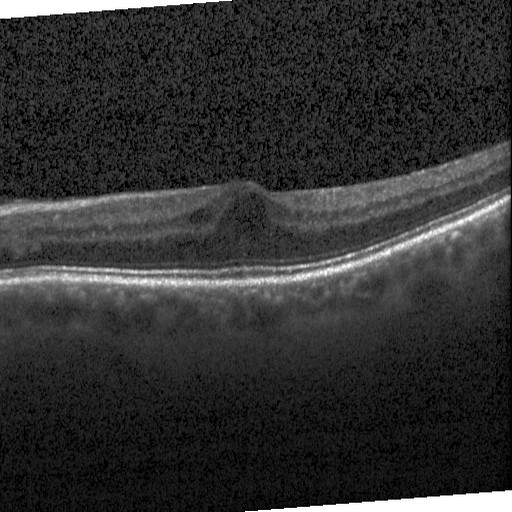

OCT finding: diabetic macular edema (DME).